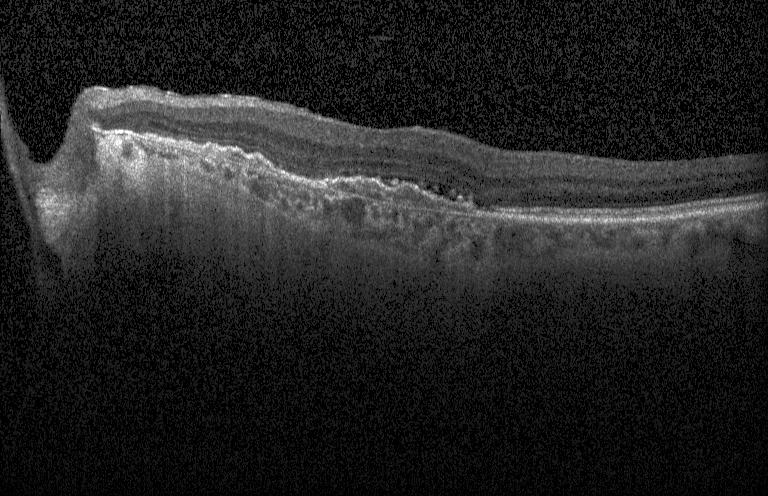 SD-OCT. OCT B-scan.
OCT finding: choroidal neovascularization (CNV).